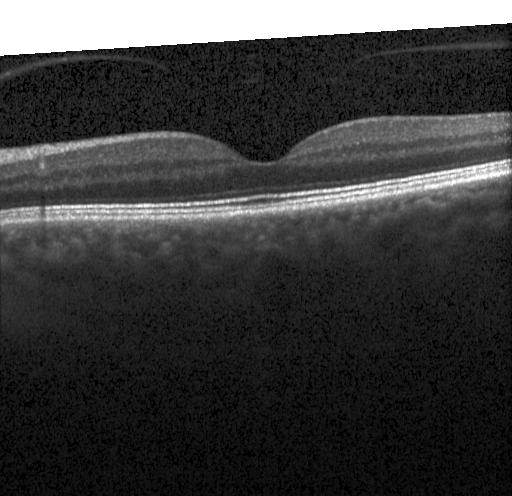 OCT B-scan showing neither choroidal neovascularization, diabetic macular edema, nor drusen.